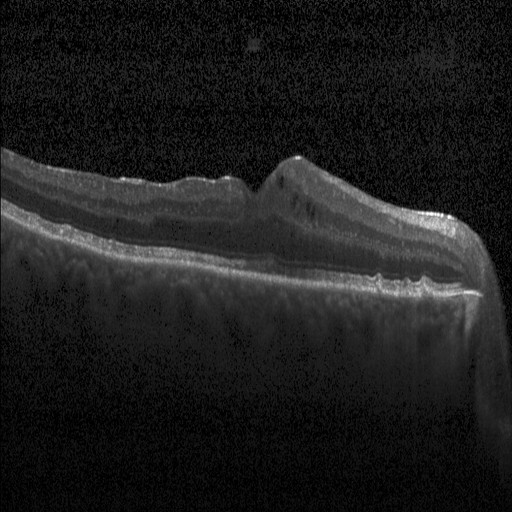

OCT B-scan, Heidelberg Spectralis OCT system.
Macular OCT: DME.